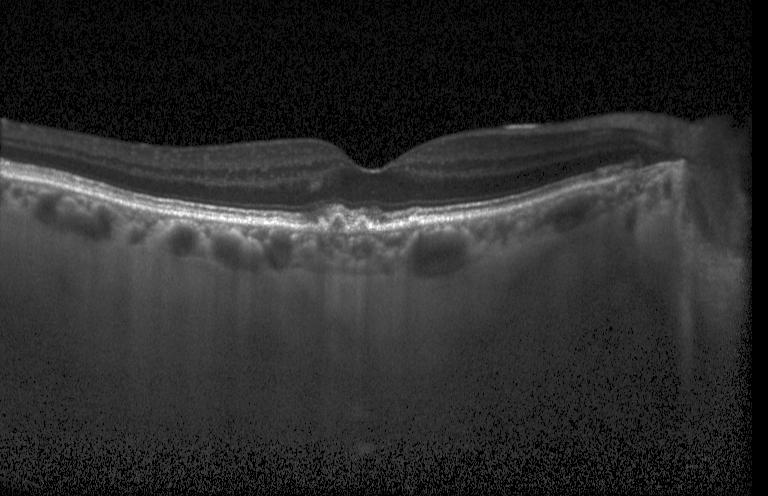 Heidelberg Spectralis OCT system. Optical coherence tomography scan. Through the macula
Diagnosis: sub-RPE drusenoid deposits.